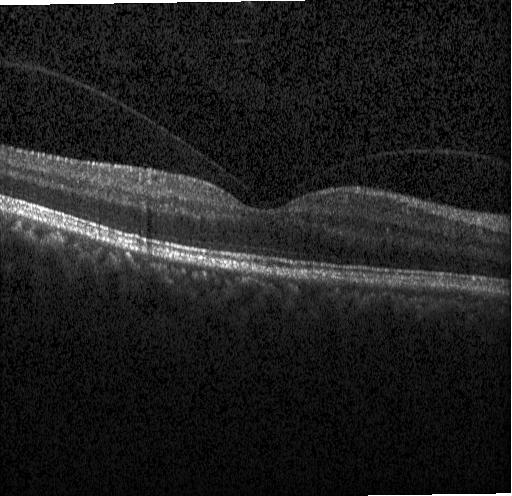 Instrument: Heidelberg Spectralis; OCT line scan. Impression: no evidence of choroidal neovascularization, diabetic macular edema, or drusen.